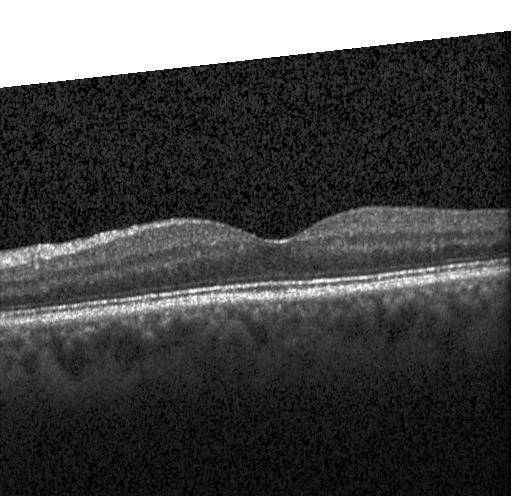 Through the macula; Heidelberg Spectralis; optical coherence tomography scan; spectral-domain optical coherence tomography.
Impression: no evidence of choroidal neovascularization, diabetic macular edema, or drusen.